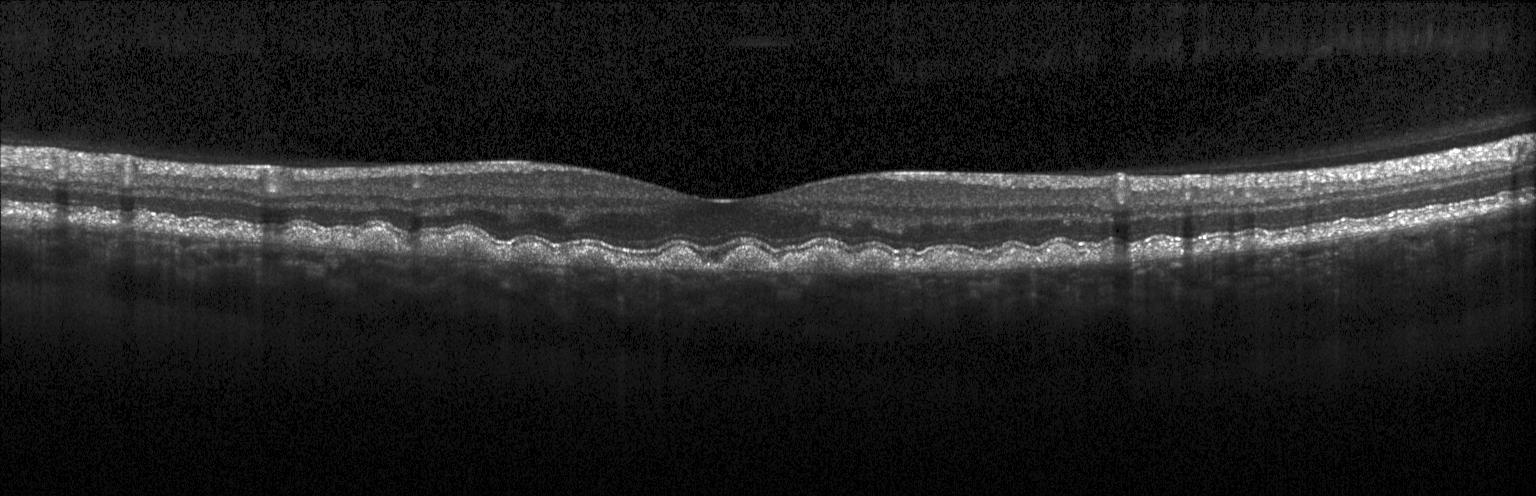

OCT finding: drusen.